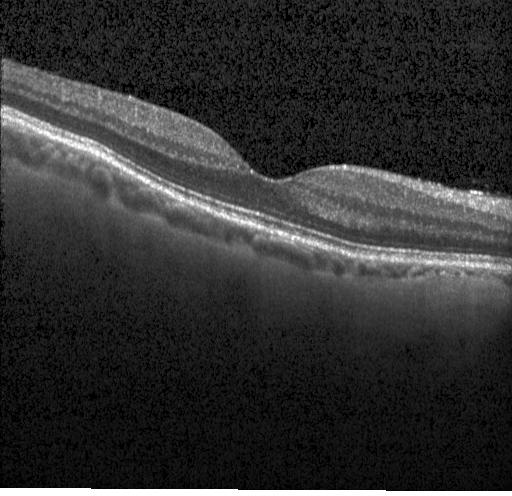 OCT finding: no evidence of choroidal neovascularization, diabetic macular edema, or drusen.